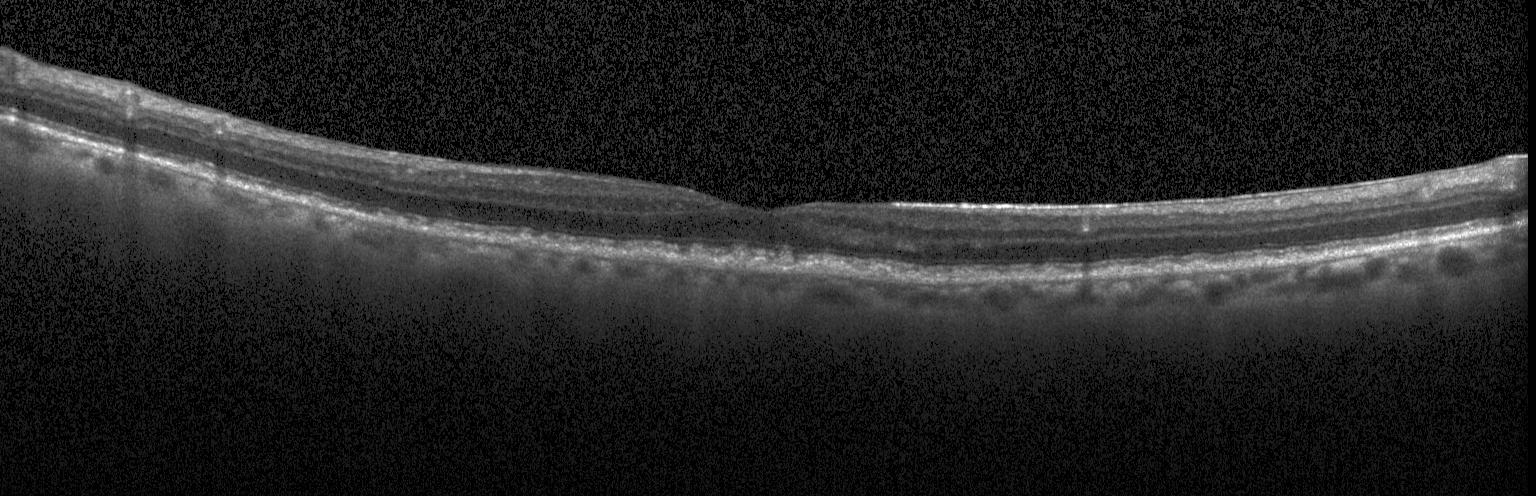
Optical coherence tomography scan. Macular scan. Spectral-domain OCT. Heidelberg Spectralis OCT system
Impression: multiple drusen.